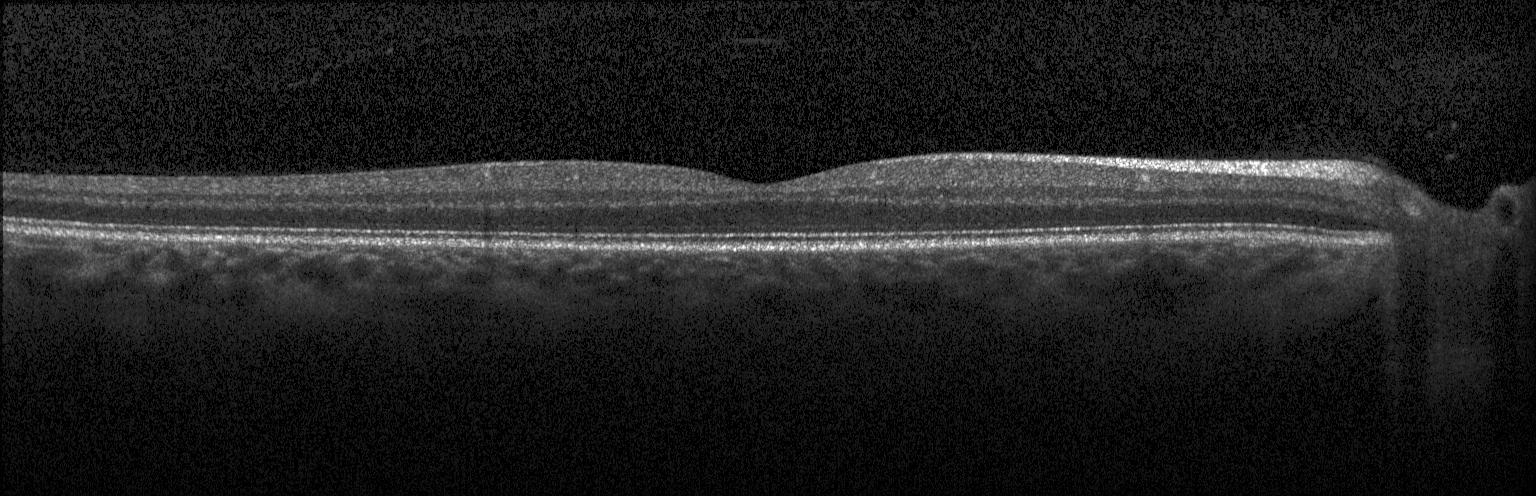
Neither choroidal neovascularization, diabetic macular edema, nor drusen.